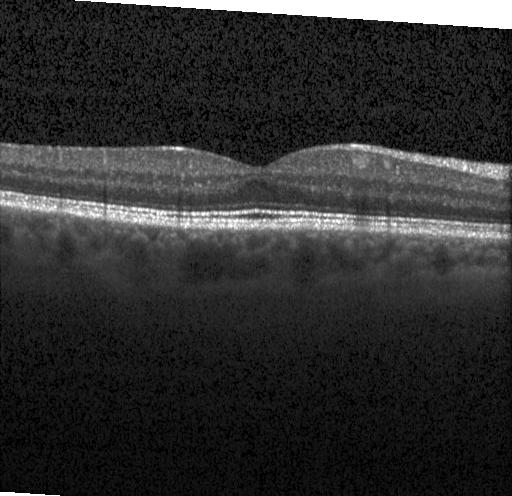
Retinal OCT cross-section — Dx: neither CNV, DME, nor drusen.